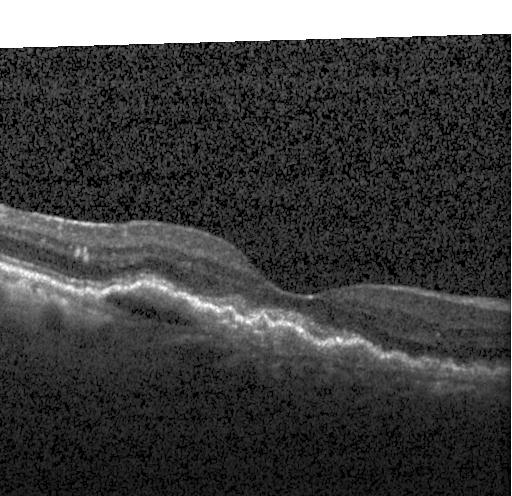
OCT line scan
Macular OCT: choroidal neovascularization.